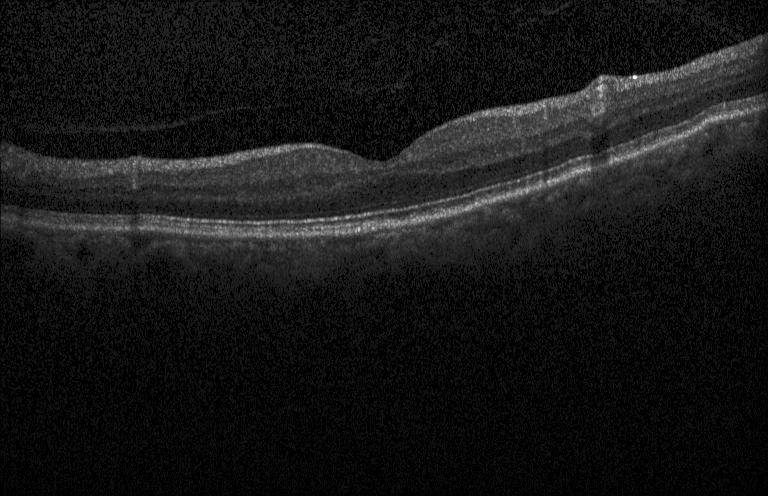
Diagnosis: no CNV, no DME, and no drusen.